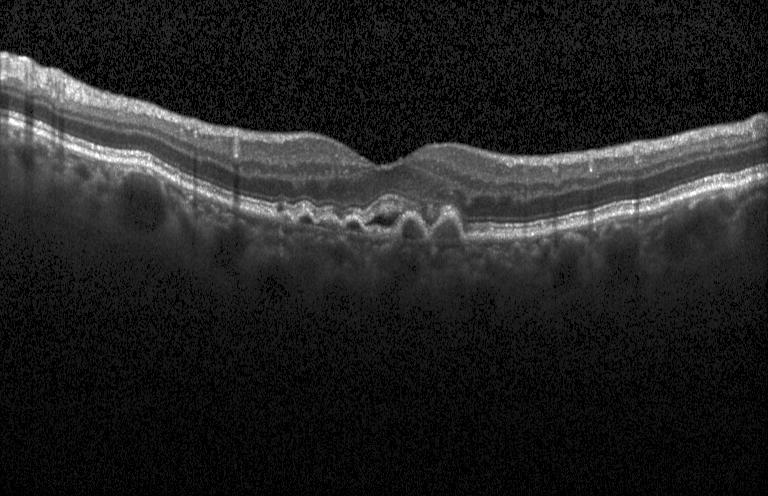

Spectral-domain optical coherence tomography · retinal OCT B-scan · fovea-centered
Finding: a choroidal neovascular membrane.